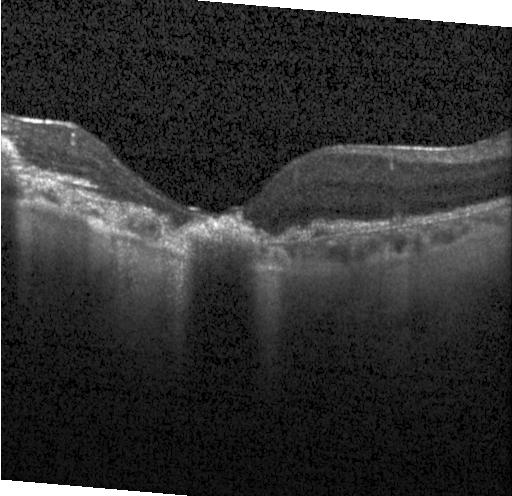
Optical coherence tomography scan. SD-OCT.
Diagnosis: a choroidal neovascular membrane.